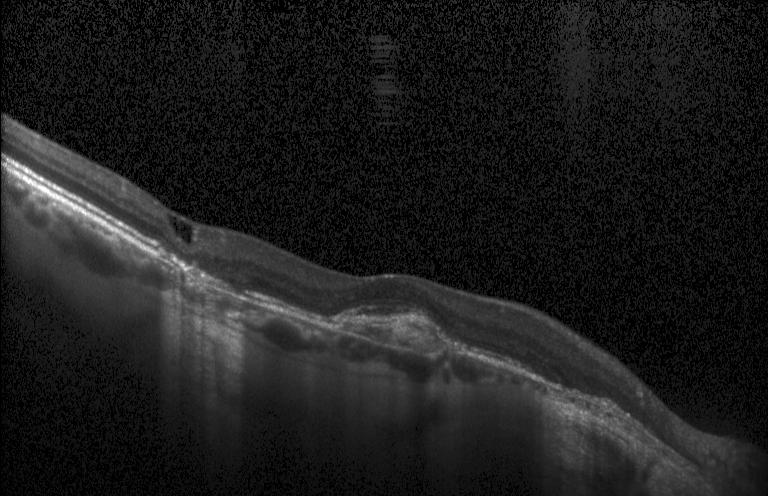
SD-OCT · retinal OCT cross-section. This B-scan demonstrates a choroidal neovascular membrane.